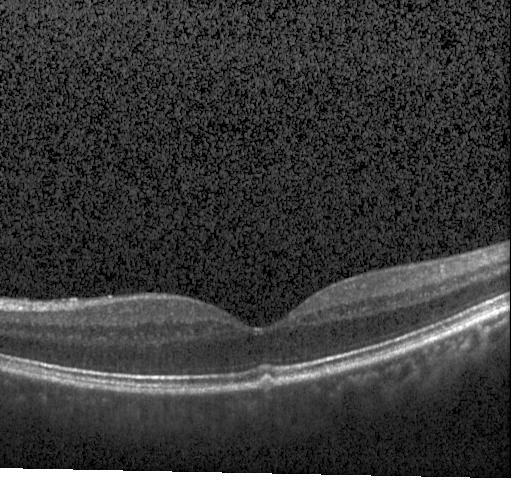
This B-scan demonstrates multiple drusen.